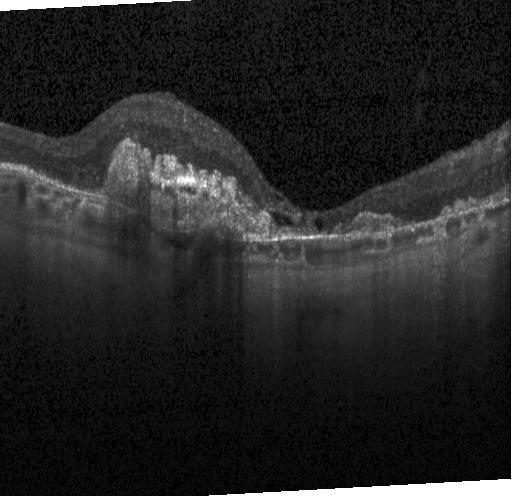
Heidelberg Spectralis OCT system · retinal OCT B-scan.
Impression: a choroidal neovascular membrane.